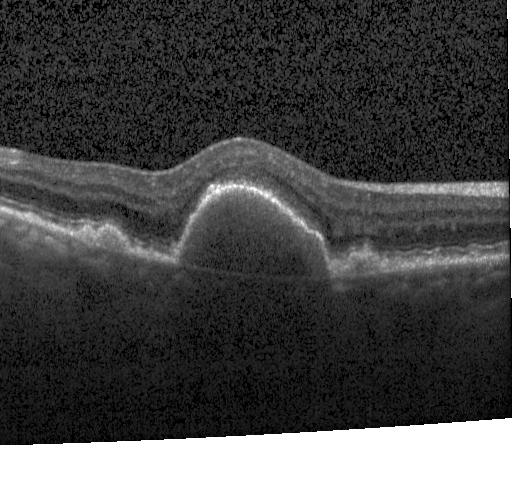
Through the macula. SD-OCT. Optical coherence tomography B-scan
Diagnosis: a choroidal neovascular membrane.